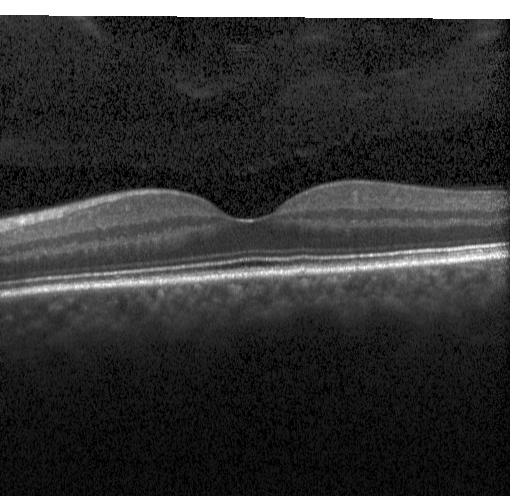
Optical coherence tomography scan; spectral-domain optical coherence tomography.
Diagnosis: no CNV, DME, or drusen.